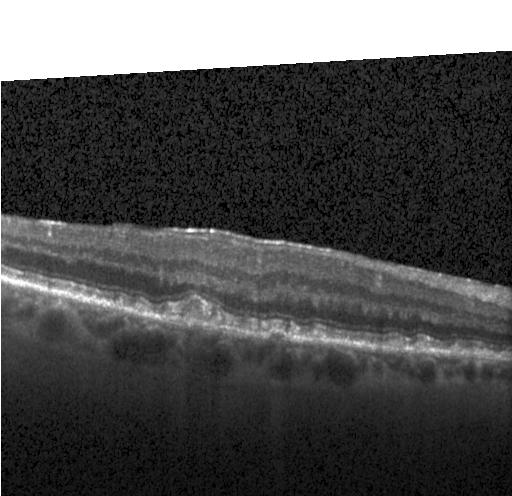
Optical coherence tomography scan — Sub-RPE drusenoid deposits.